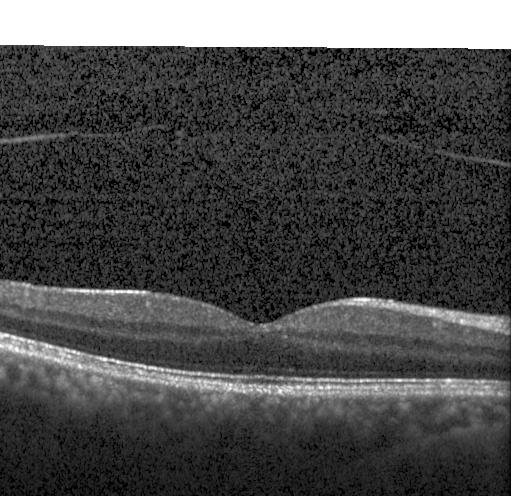

OCT line scan
Impression: no choroidal neovascularization, no diabetic macular edema, and no drusen.